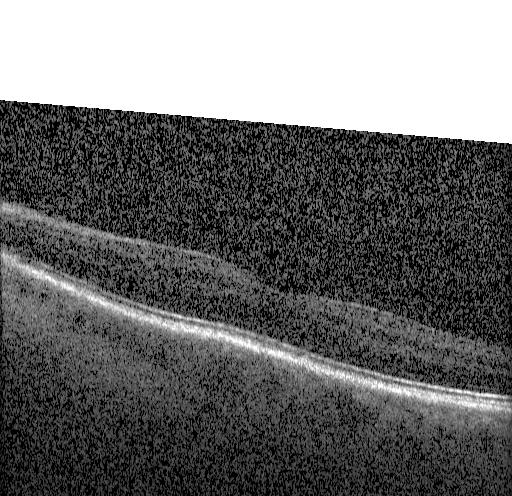

Macular OCT: neither choroidal neovascularization, diabetic macular edema, nor drusen.